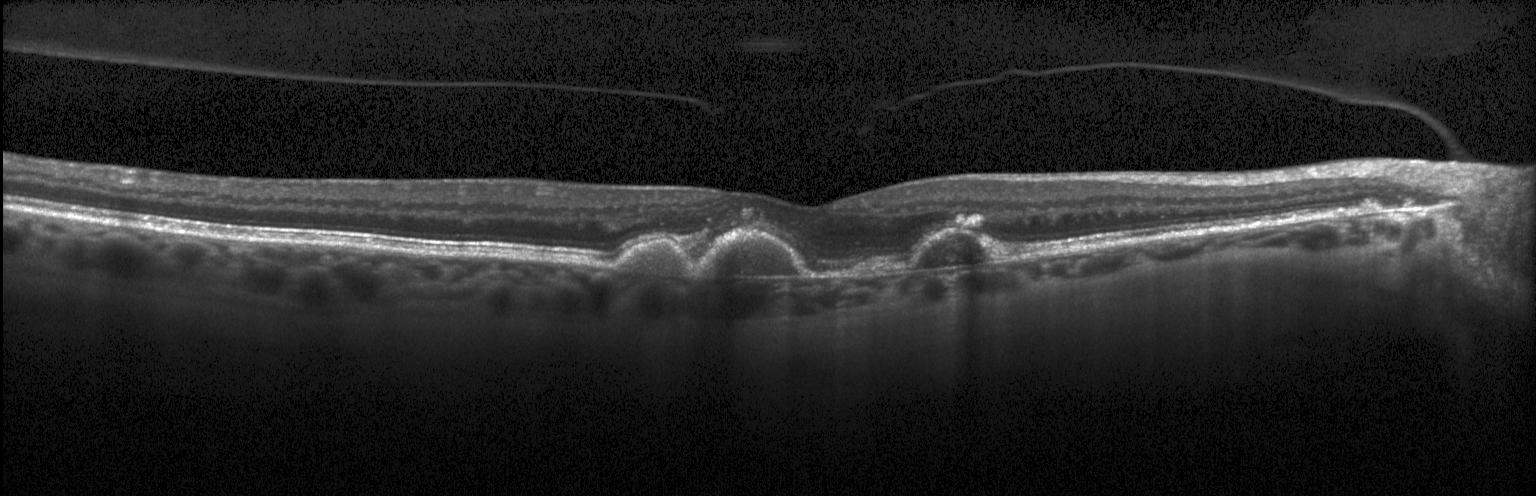 Diagnosis: CNV.